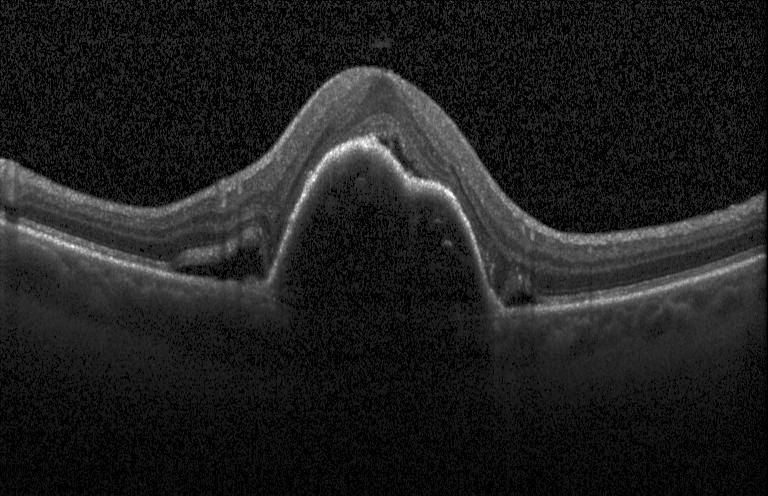 Spectral-domain OCT · centered on the fovea · instrument: Heidelberg Spectralis · retinal OCT cross-section. Diagnosis: a choroidal neovascular membrane.